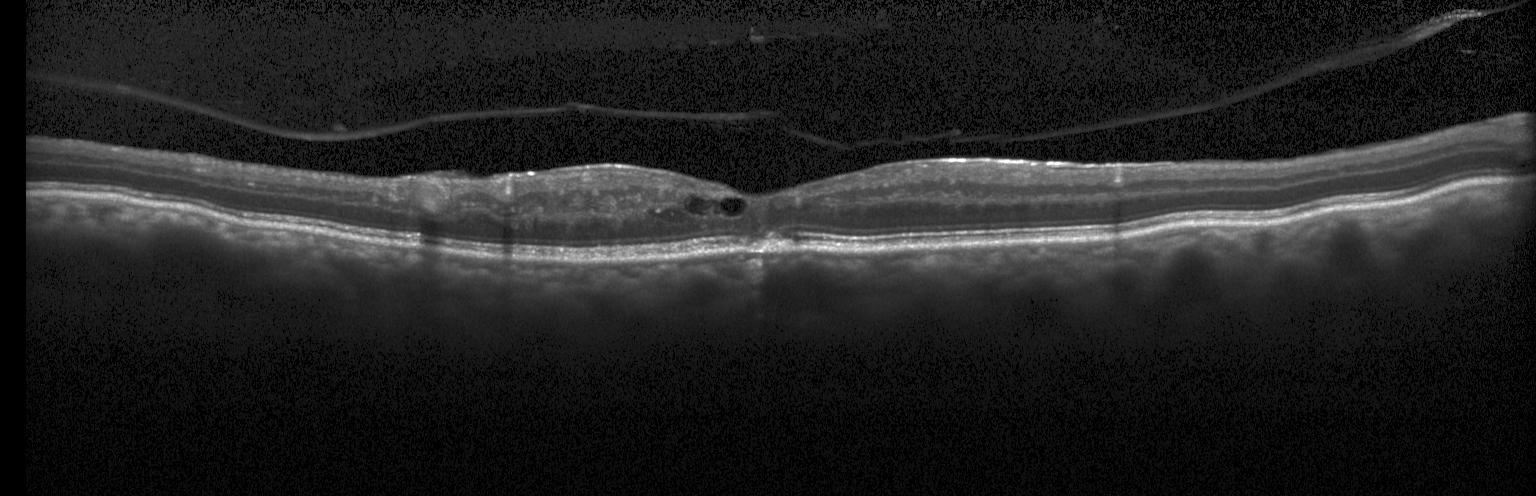
Diabetic macular edema (DME).